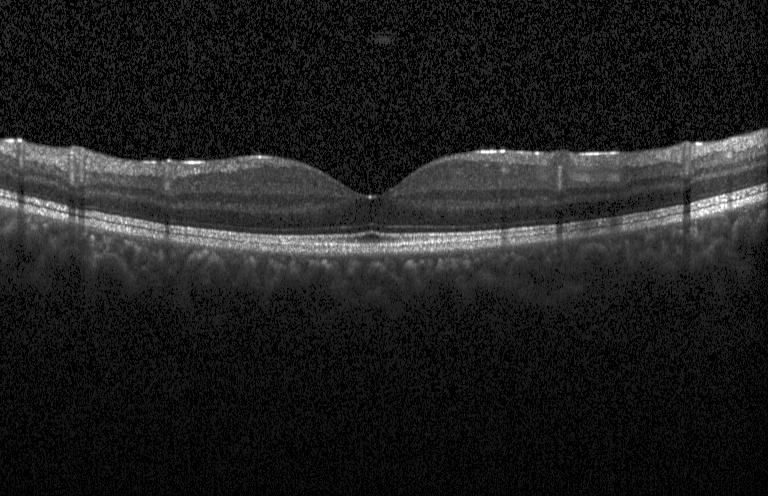

Horizontal scan through the fovea. SD-OCT. OCT line scan.
Impression: no CNV, DME, or drusen.